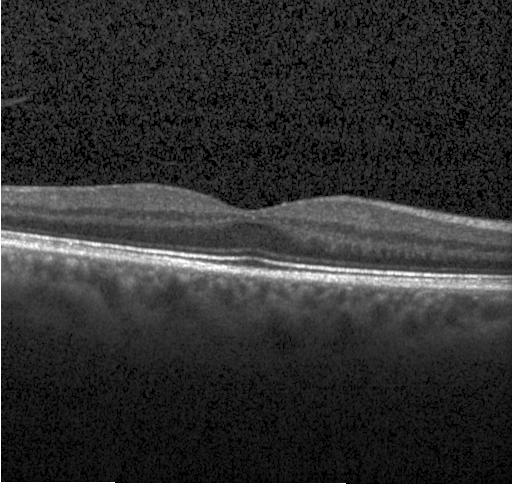
Spectral-domain OCT B-scan: no evidence of choroidal neovascularization, diabetic macular edema, or drusen.